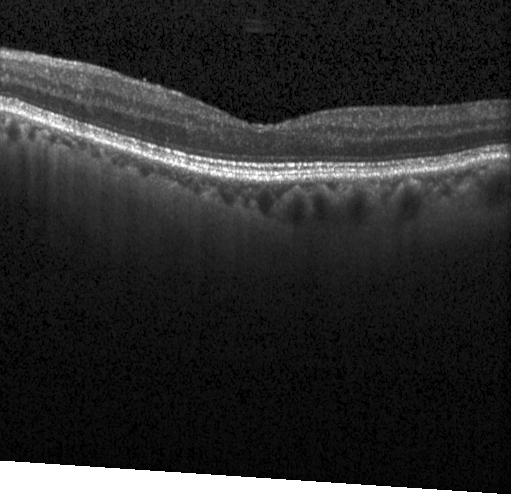

Acquired on a Heidelberg Spectralis · fovea-centered · optical coherence tomography scan · SD-OCT.
Diagnosis: neither choroidal neovascularization, diabetic macular edema, nor drusen.